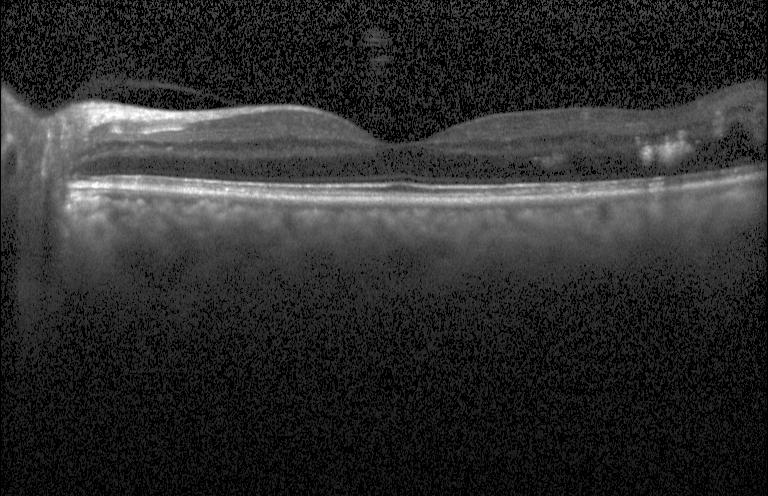
Optical coherence tomography scan, spectral-domain OCT. Impression: diabetic macular edema.